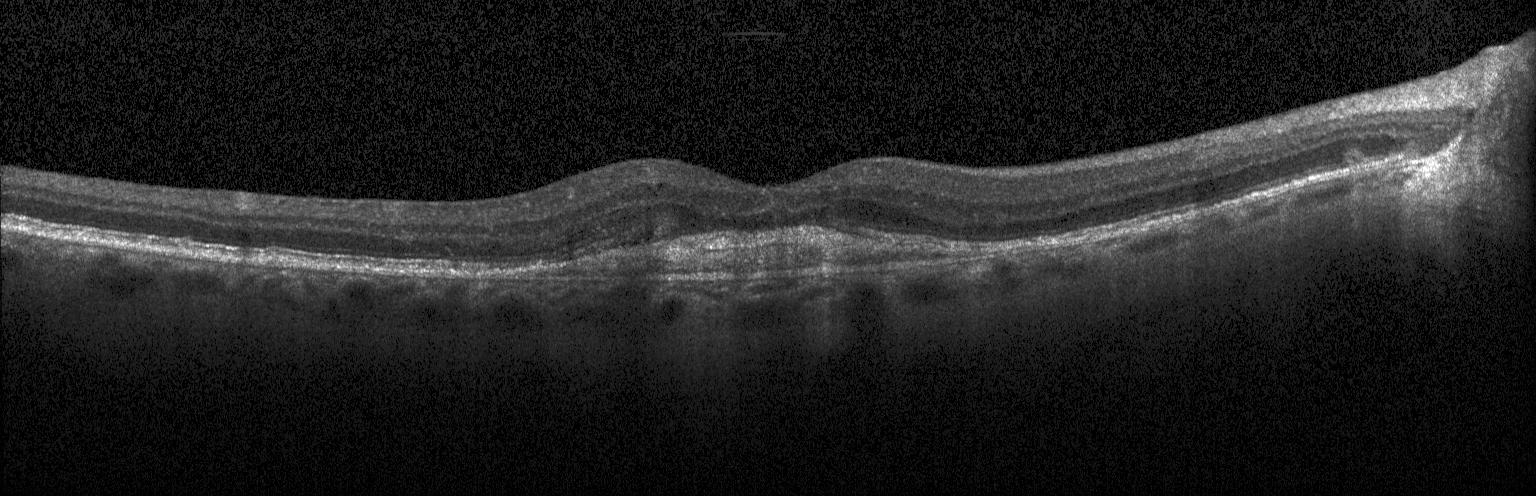

Instrument: Heidelberg Spectralis, optical coherence tomography B-scan. A choroidal neovascular membrane.